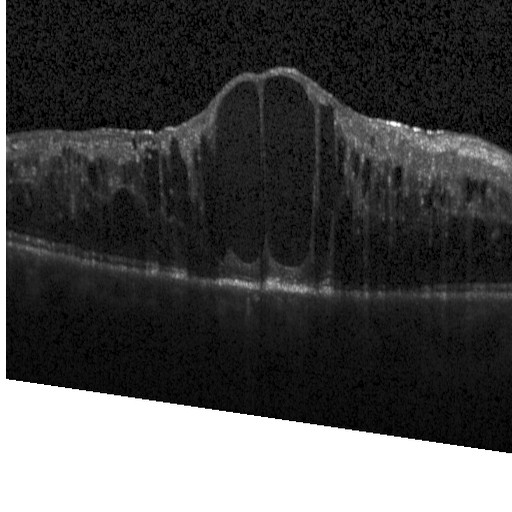
Dx: diabetic macular edema.